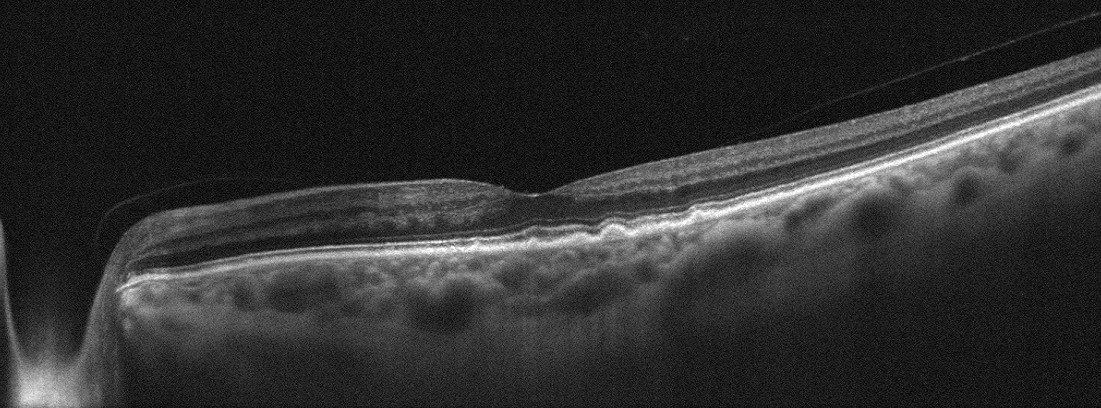
Optical coherence tomography scan. Assessment: age-related macular degeneration.